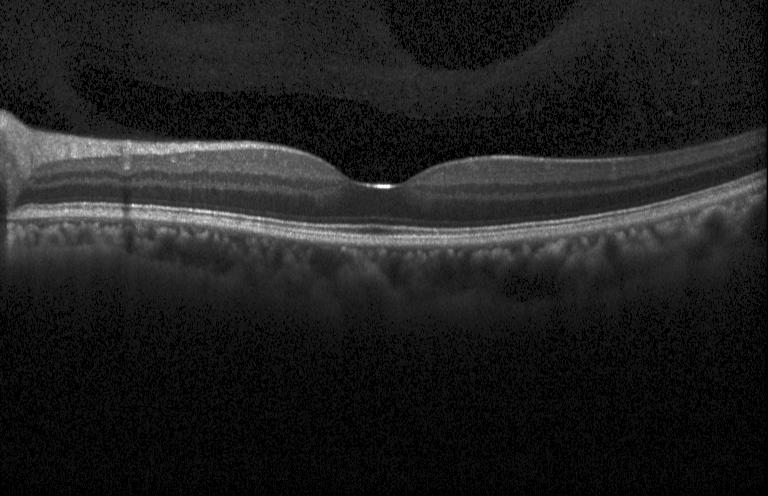 Assessment: no choroidal neovascularization, no diabetic macular edema, and no drusen.